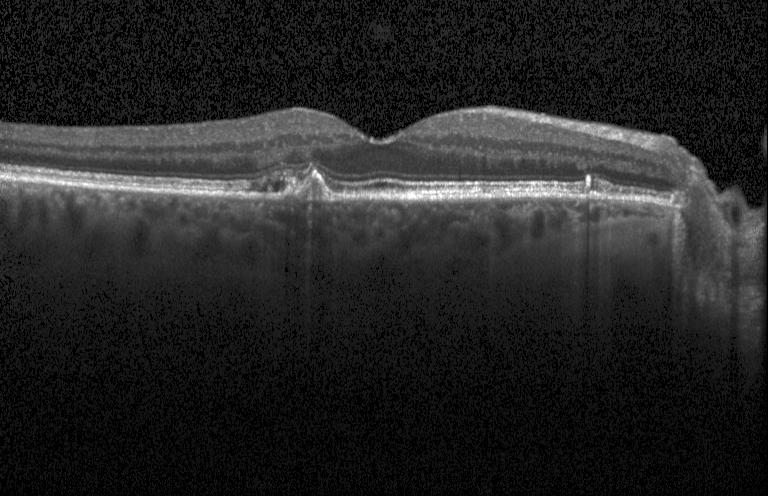

Retinal OCT B-scan · Heidelberg Spectralis · through the macula — Impression: a choroidal neovascular membrane.